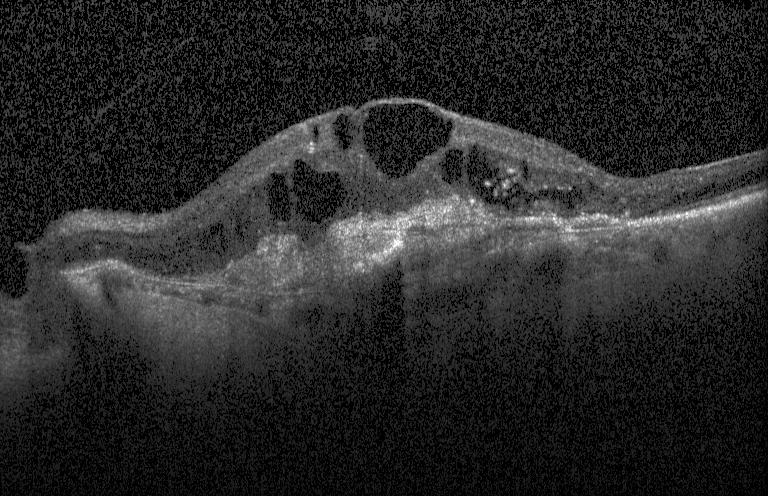
Heidelberg Spectralis OCT system · spectral-domain OCT · fovea-centered · OCT line scan.
This B-scan demonstrates a choroidal neovascular membrane.